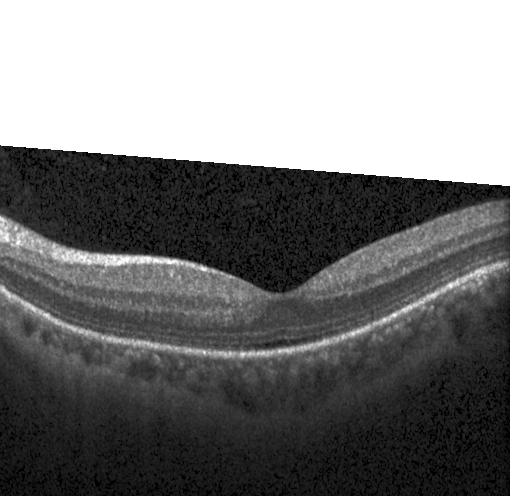
Diagnosis: no evidence of choroidal neovascularization, diabetic macular edema, or drusen.